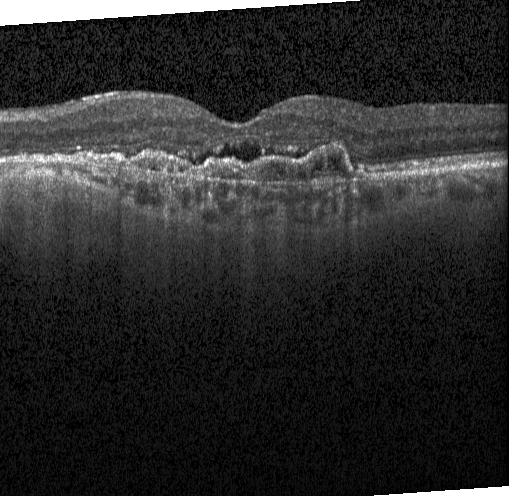 A choroidal neovascular membrane.